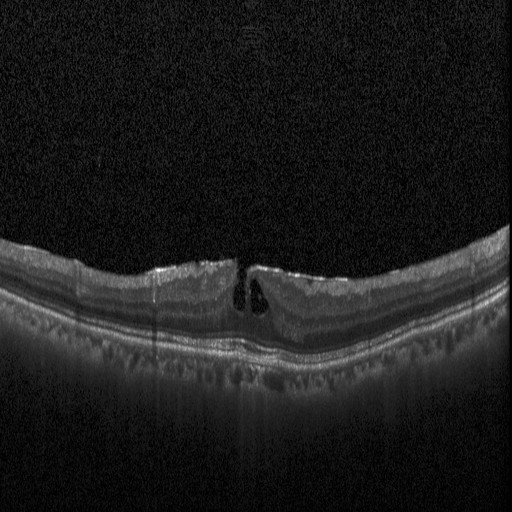

OCT B-scan · instrument: Heidelberg Spectralis · centered on the fovea — The scan shows DME.